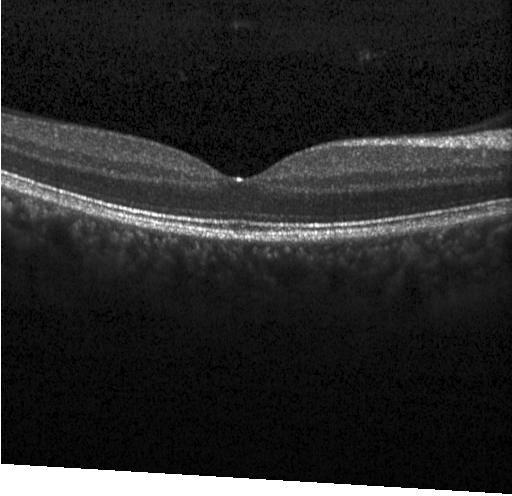

OCT line scan; acquired on a Heidelberg Spectralis. The scan shows neither CNV, DME, nor drusen.